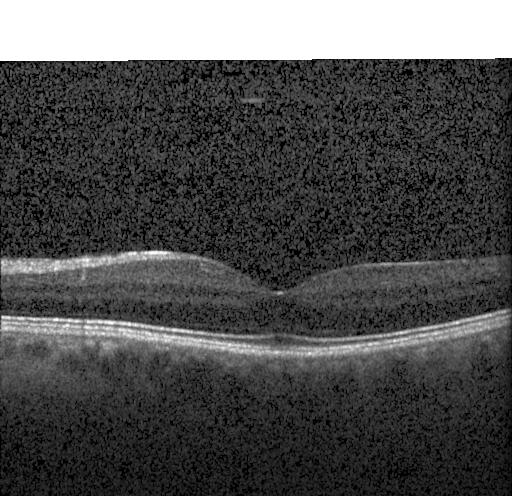 Spectral-domain OCT. Optical coherence tomography scan. Heidelberg Spectralis OCT system. Horizontal scan through the fovea
Macular OCT: no evidence of choroidal neovascularization, diabetic macular edema, or drusen.